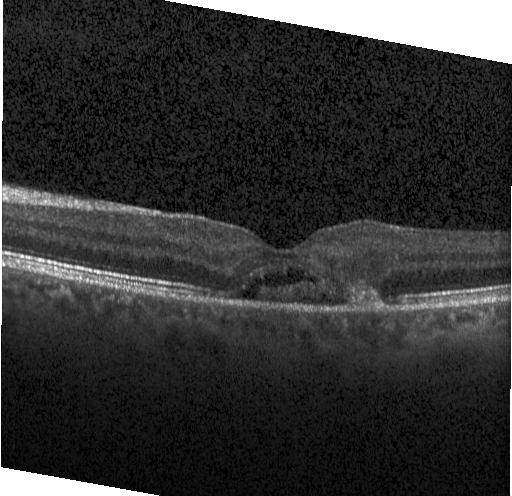 Horizontal scan through the fovea. Heidelberg Spectralis. Spectral-domain optical coherence tomography. Optical coherence tomography scan
Dx: a choroidal neovascular membrane.